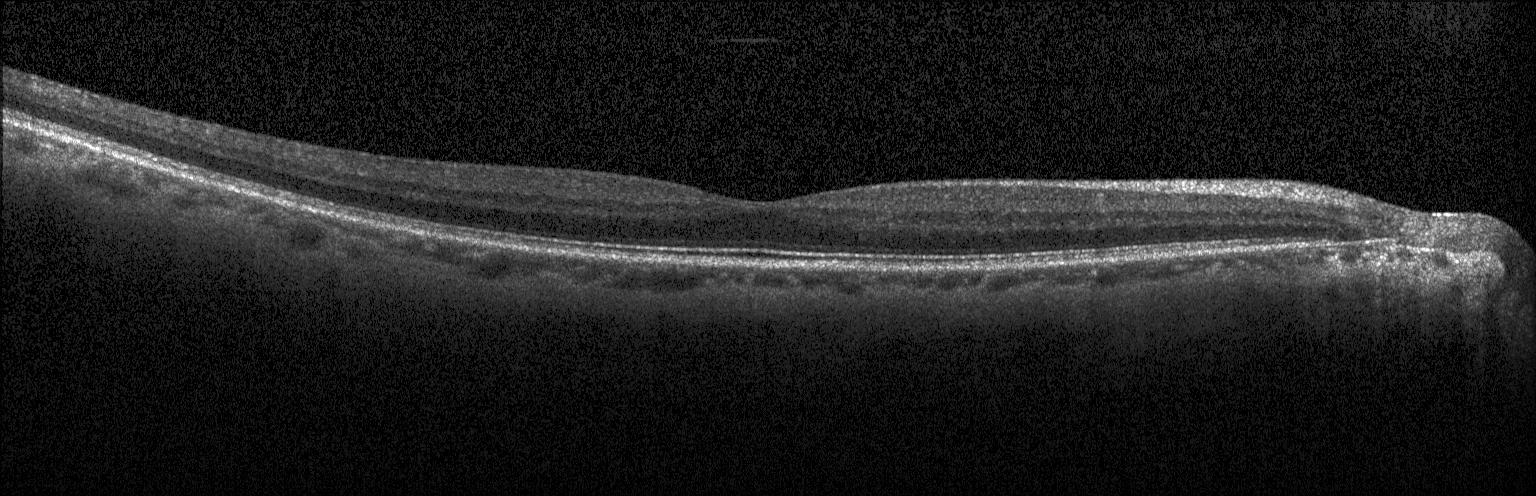

No CNV, no DME, and no drusen.